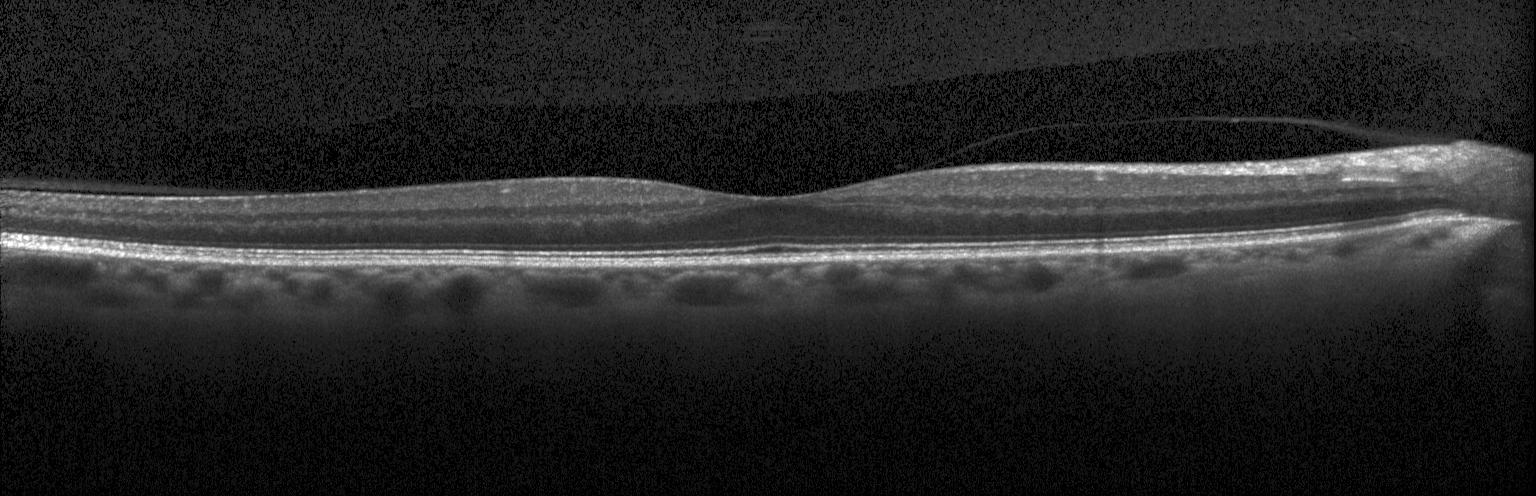

Retinal OCT B-scan — Macular OCT: no CNV, no DME, and no drusen.